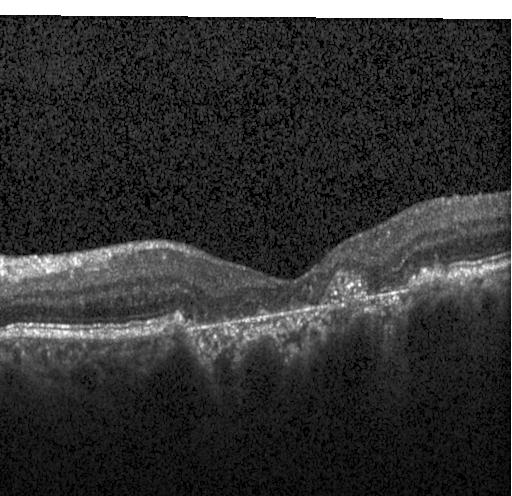 Impression: CNV.